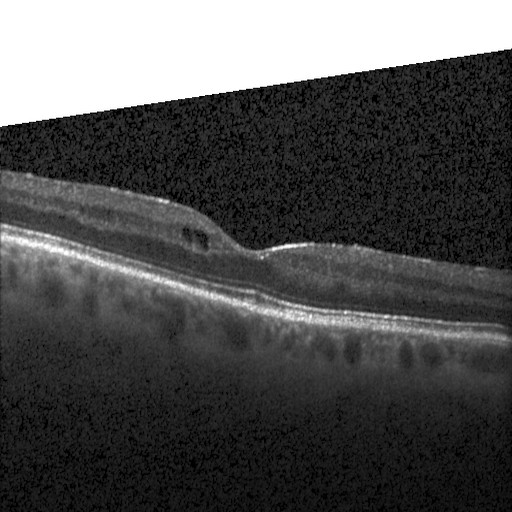
Horizontal scan through the fovea, optical coherence tomography scan, spectral-domain optical coherence tomography, Heidelberg Spectralis. Finding: diabetic macular edema.